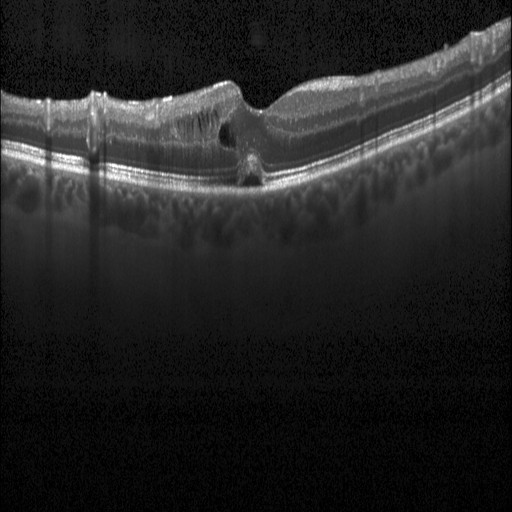
Macular OCT demonstrating diabetic macular edema (DME).